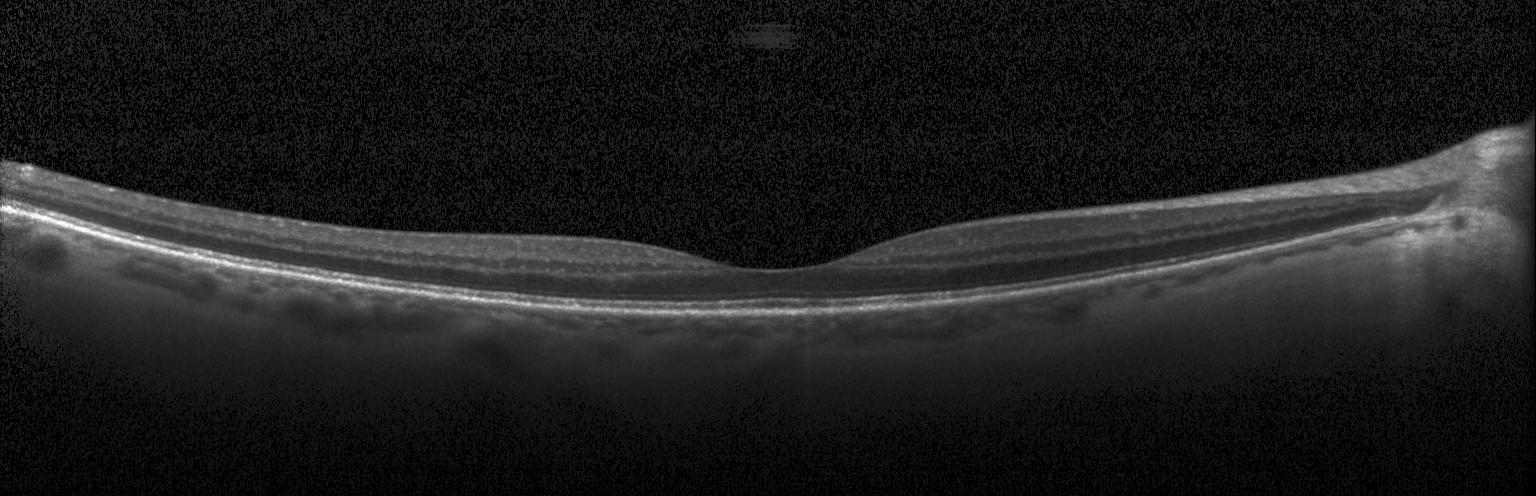
Acquired on a Heidelberg Spectralis · centered on the fovea · spectral-domain OCT · optical coherence tomography B-scan
Finding: no choroidal neovascularization, no diabetic macular edema, and no drusen.